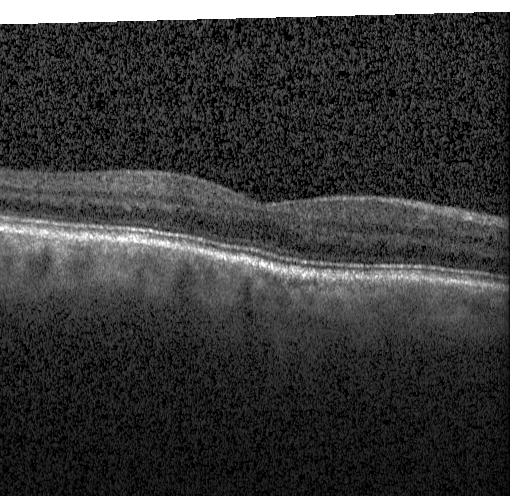
Optical coherence tomography B-scan. Finding: no choroidal neovascularization, no diabetic macular edema, and no drusen.